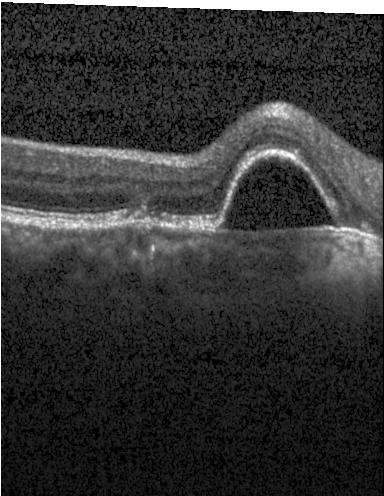 OCT B-scan — Dx: a choroidal neovascular membrane.